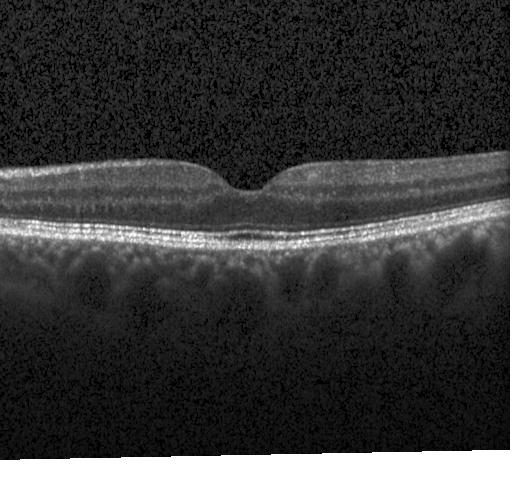
Optical coherence tomography scan. Spectral-domain OCT. Instrument: Heidelberg Spectralis — This B-scan demonstrates neither choroidal neovascularization, diabetic macular edema, nor drusen.